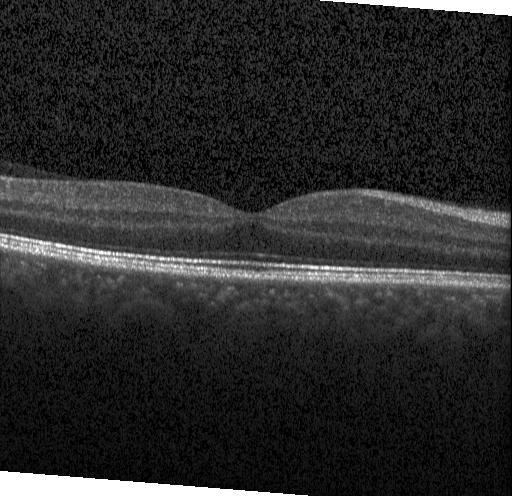
Retinal OCT cross-section · fovea-centered.
OCT finding: no CNV, DME, or drusen.